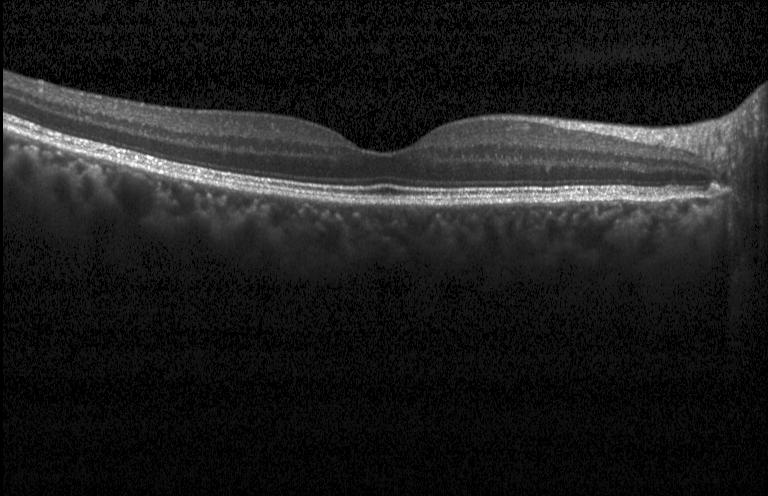
OCT B-scan showing no CNV, DME, or drusen.